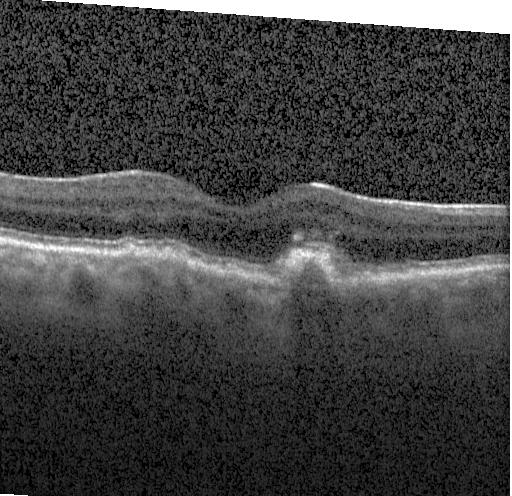 Macular OCT demonstrating drusen.